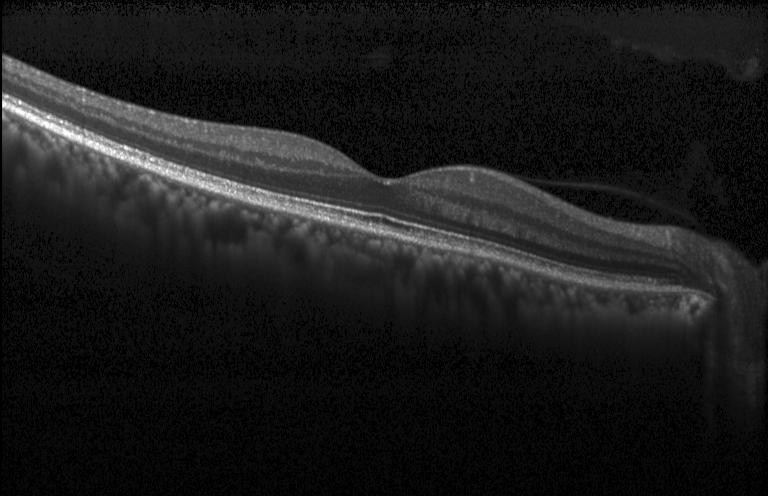
Diagnosis: no CNV, no DME, and no drusen.